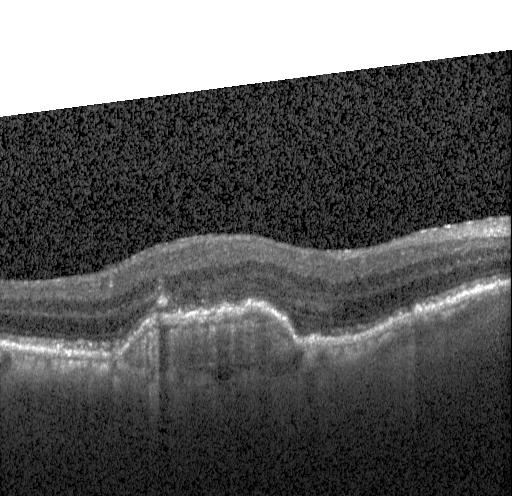 OCT line scan
Impression: choroidal neovascularization (CNV).